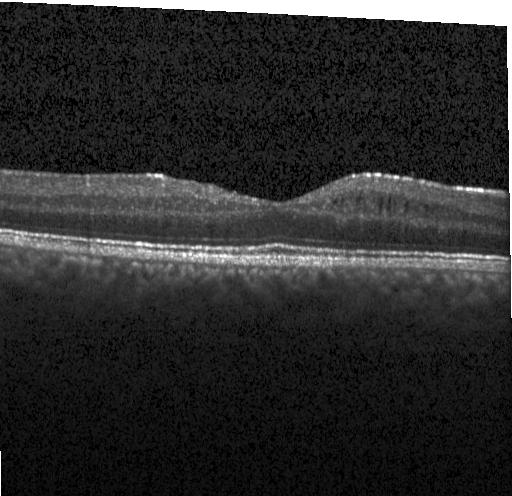 Impression: diabetic macular edema.